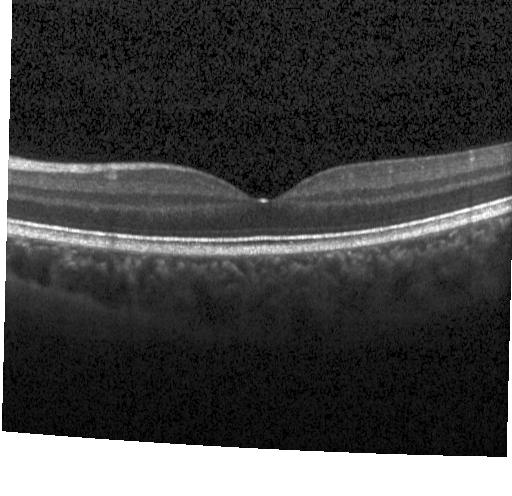 Retinal OCT B-scan — Impression: no evidence of choroidal neovascularization, diabetic macular edema, or drusen.